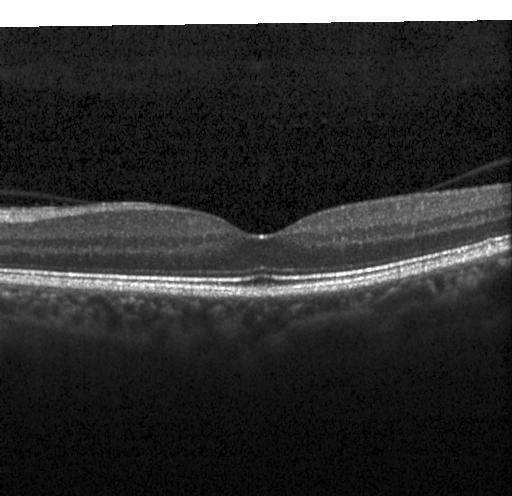

Impression: no CNV, DME, or drusen.